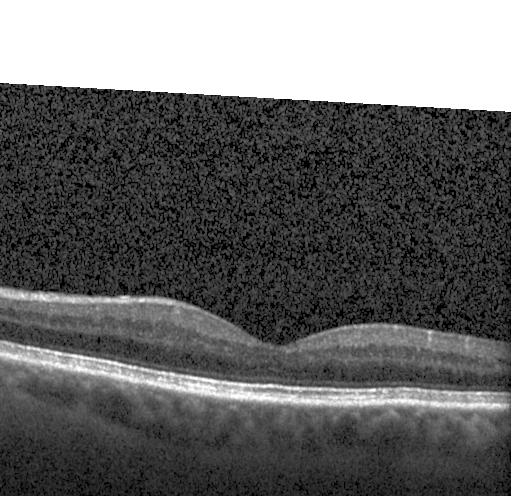
Spectral-domain OCT B-scan: neither choroidal neovascularization, diabetic macular edema, nor drusen.